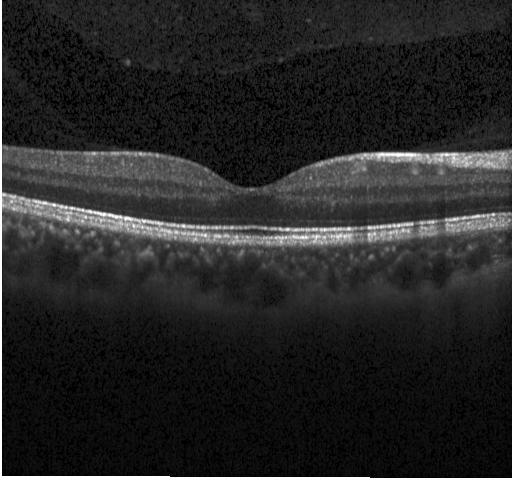
Dx: no evidence of choroidal neovascularization, diabetic macular edema, or drusen.